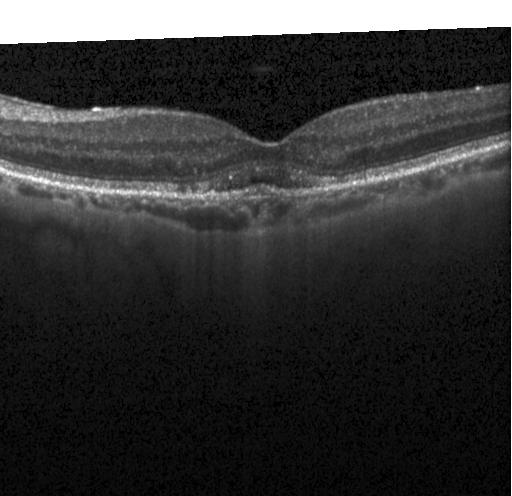

Retinal OCT B-scan. Macular OCT: a choroidal neovascular membrane.